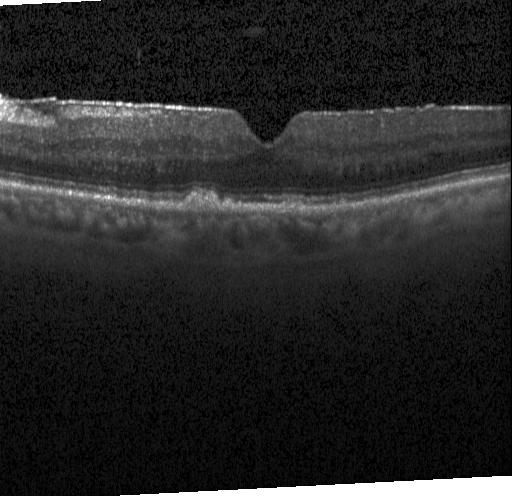

OCT line scan — Diagnosis: drusen.